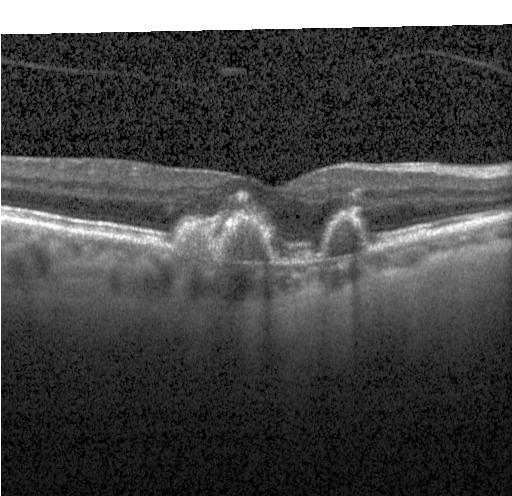

Impression: choroidal neovascularization.